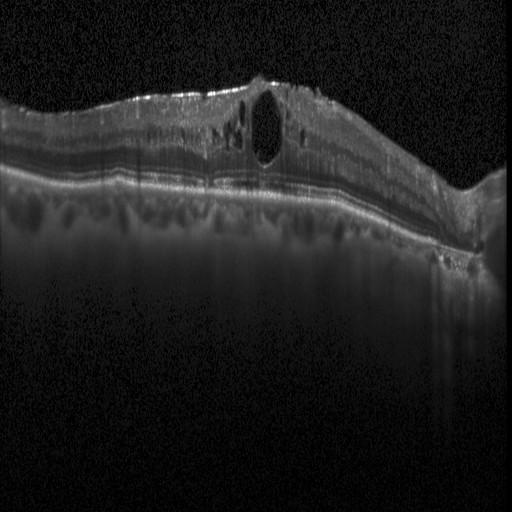 OCT finding: diabetic macular edema (DME).